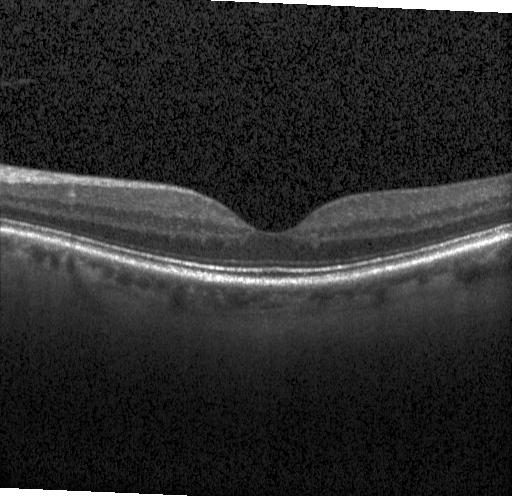

Instrument: Heidelberg Spectralis. Horizontal scan through the fovea. Optical coherence tomography scan — Dx: no evidence of choroidal neovascularization, diabetic macular edema, or drusen.